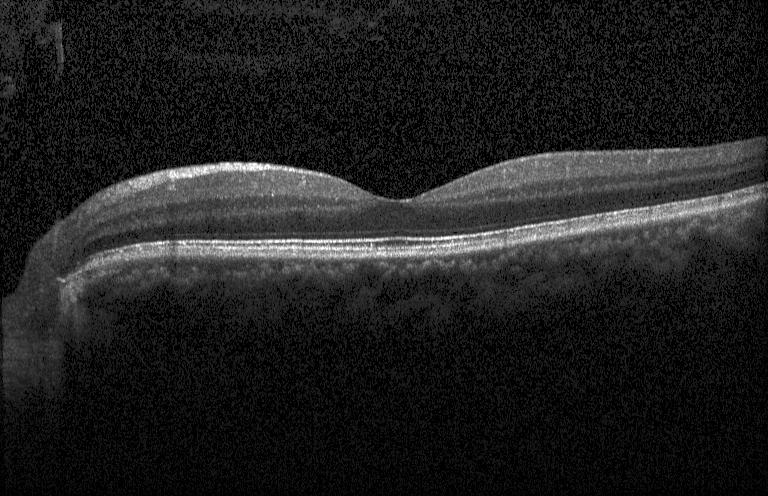
Impression: no evidence of choroidal neovascularization, diabetic macular edema, or drusen.